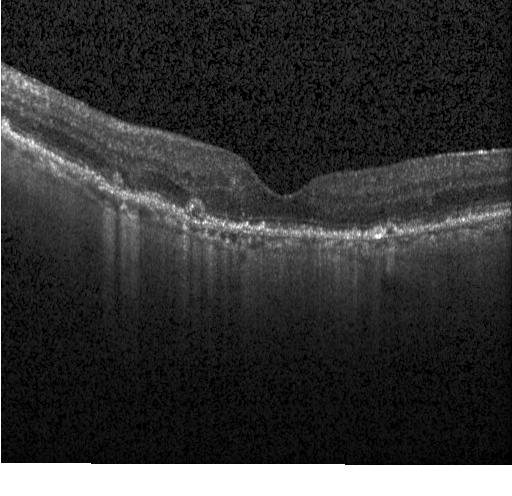 Spectral-domain optical coherence tomography, optical coherence tomography B-scan, fovea-centered — Impression: a choroidal neovascular membrane.